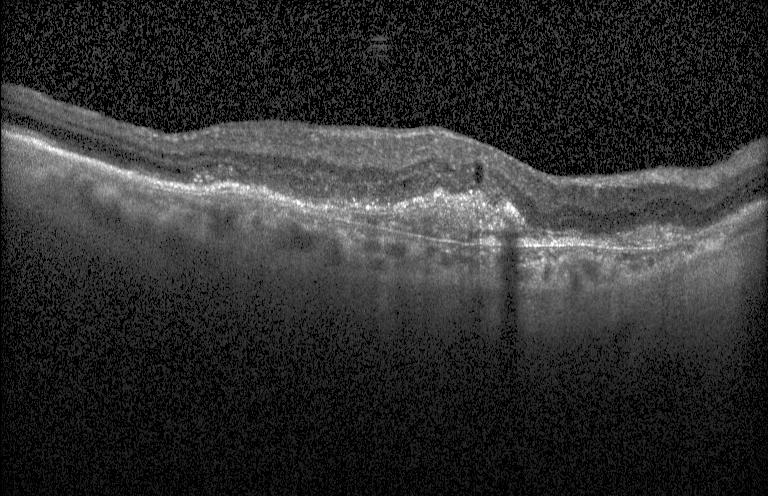
Macular scan; Heidelberg Spectralis; OCT line scan; spectral-domain OCT
Macular OCT: CNV.